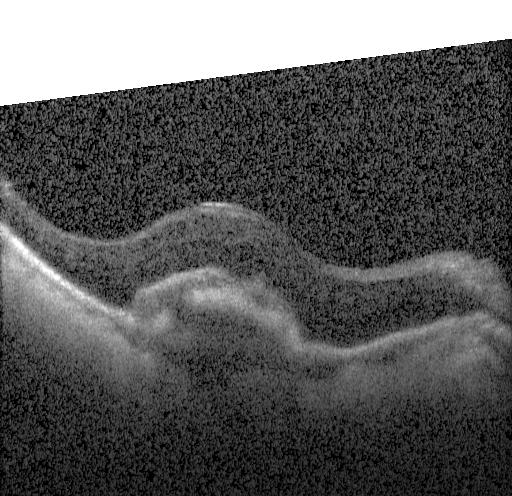 Through the macula, Heidelberg Spectralis, retinal OCT B-scan
Impression: CNV.